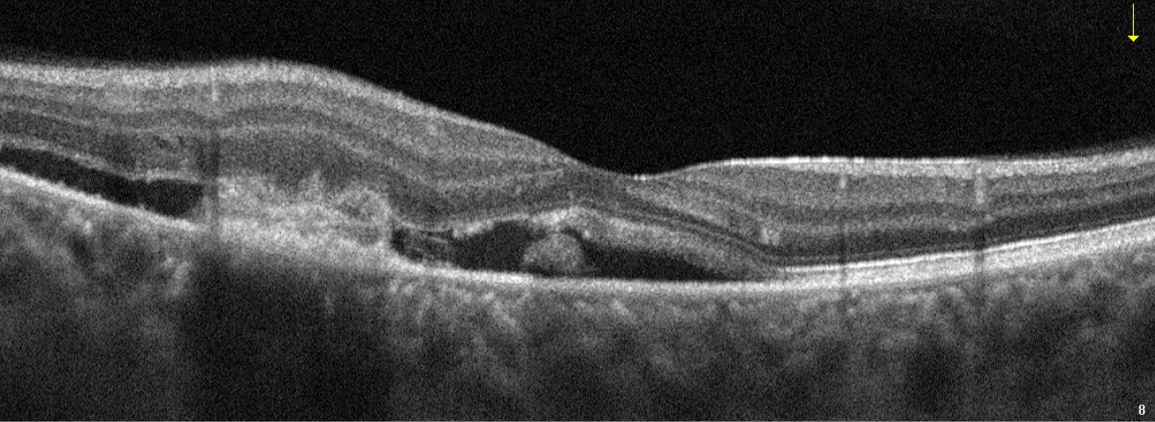 Impression: age-related macular degeneration.